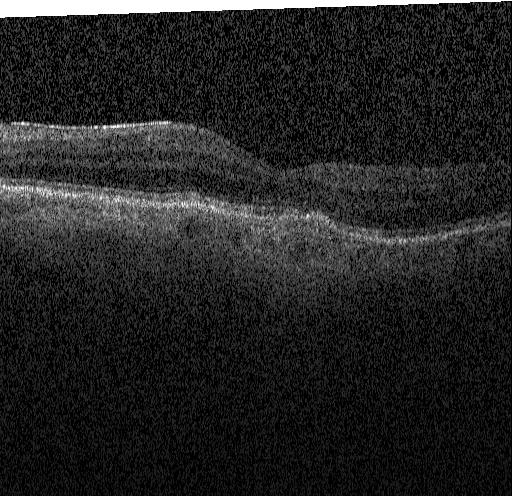

Centered on the fovea · OCT B-scan. This B-scan demonstrates a choroidal neovascular membrane.